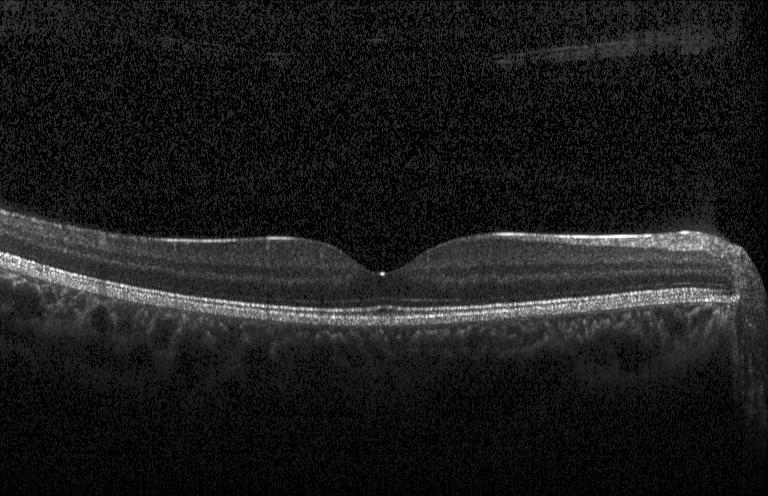
Macular OCT demonstrating neither CNV, DME, nor drusen.